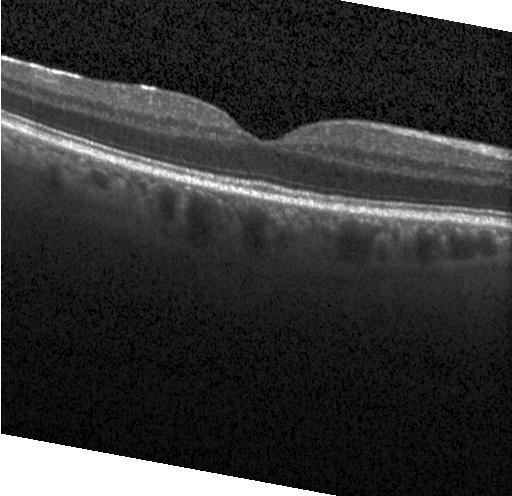
Macular OCT: no choroidal neovascularization, no diabetic macular edema, and no drusen.